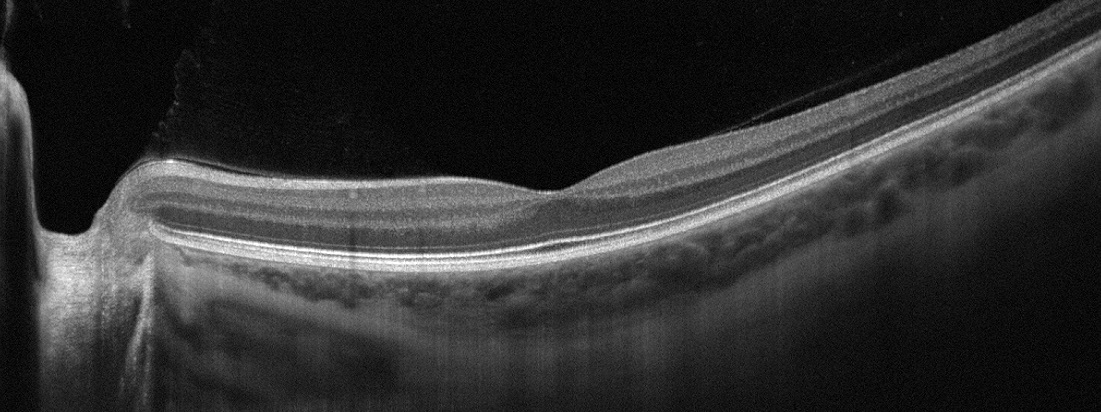 Instrument: Optovue Avanti RTVue XR. Macular scan. Optical coherence tomography scan — OCT finding: absence of AMD, DME, ERM, RAO, RVO, and vitreomacular interface disease.